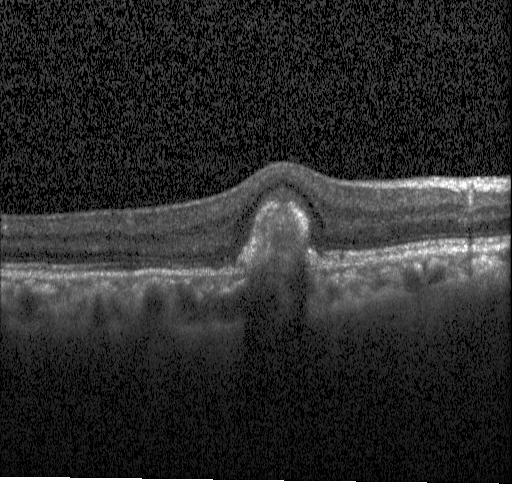

OCT B-scan — Finding: a choroidal neovascular membrane.